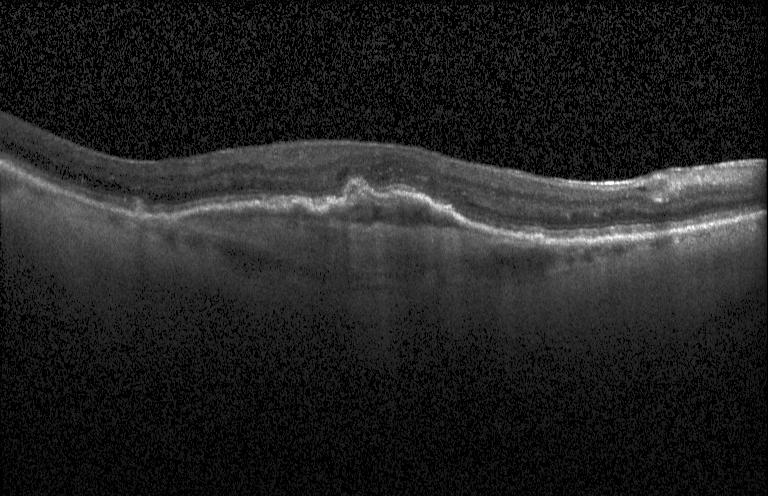

SD-OCT; retinal OCT B-scan; through the macula
Finding: a choroidal neovascular membrane.